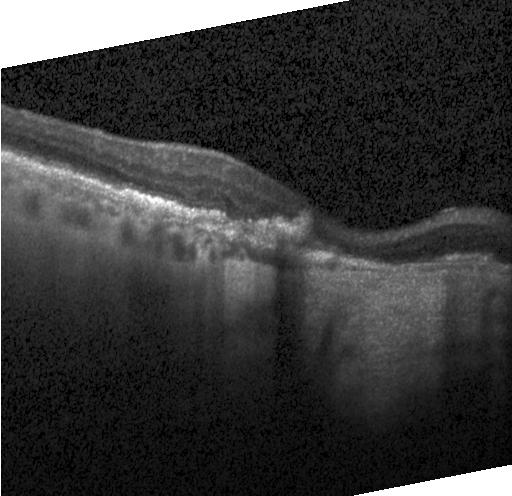 Retinal OCT cross-section showing a choroidal neovascular membrane.